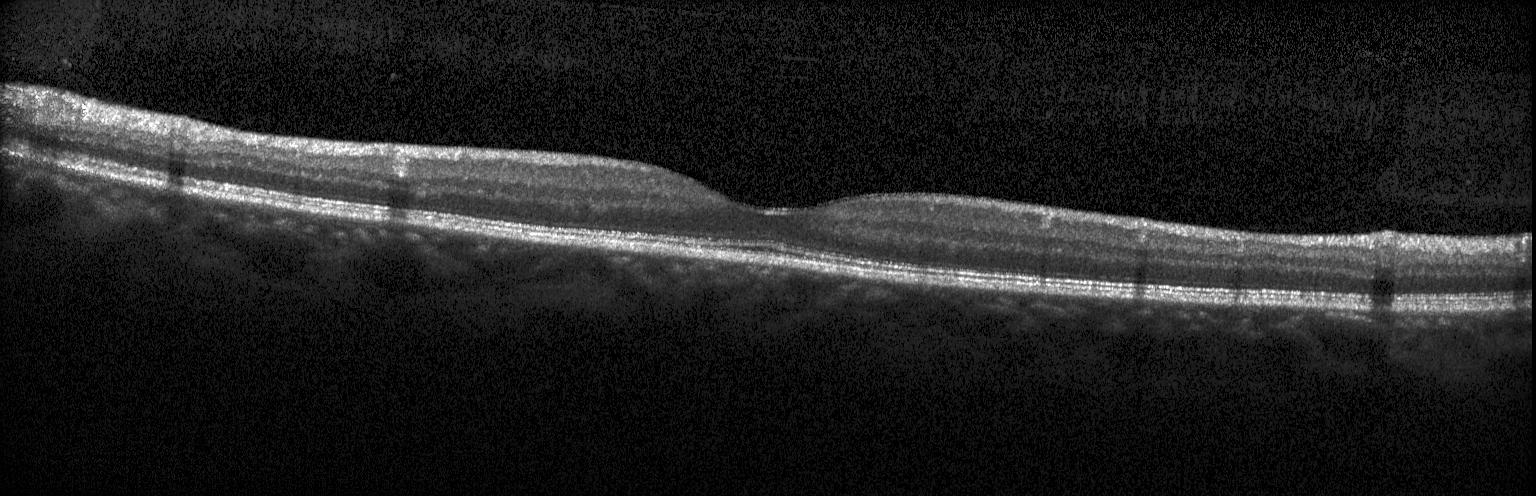

Retinal OCT cross-section.
Impression: no CNV, DME, or drusen.